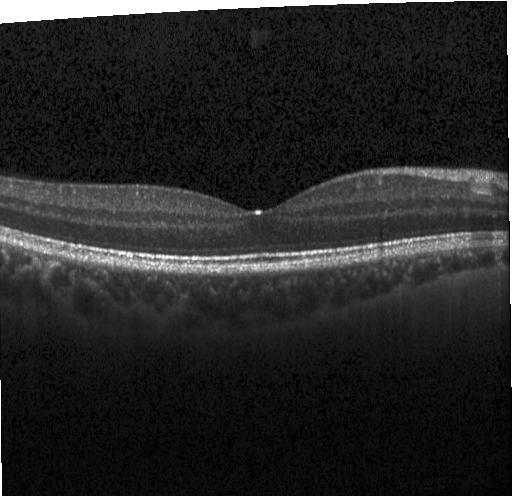

OCT line scan.
This B-scan demonstrates no evidence of choroidal neovascularization, diabetic macular edema, or drusen.